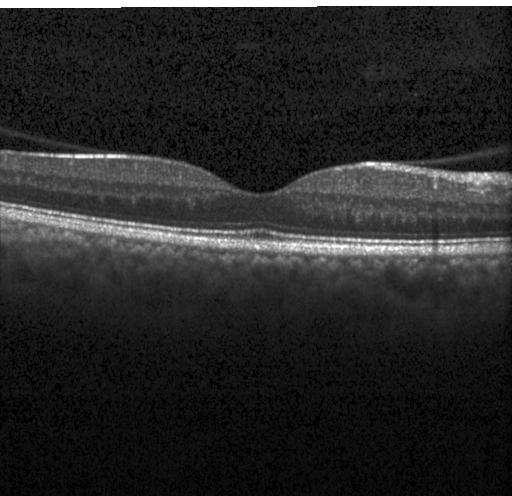
Spectral-domain OCT · optical coherence tomography scan. This B-scan demonstrates no evidence of choroidal neovascularization, diabetic macular edema, or drusen.